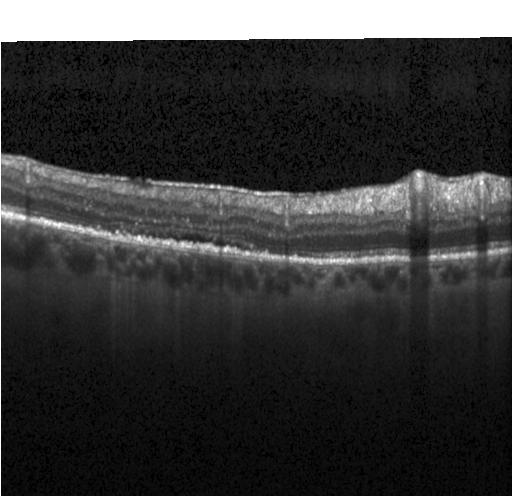

Dx: choroidal neovascularization (CNV).